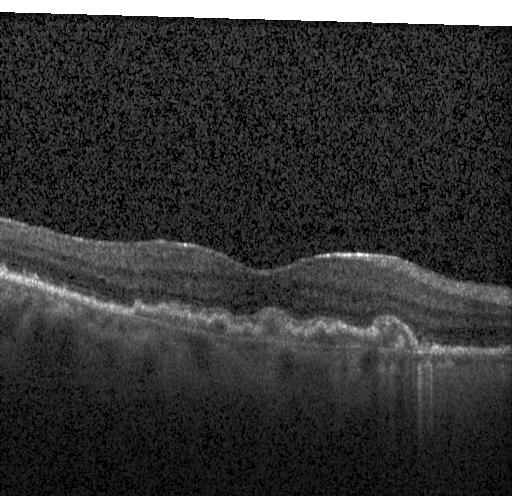

Through the macula; retinal OCT B-scan. A choroidal neovascular membrane.